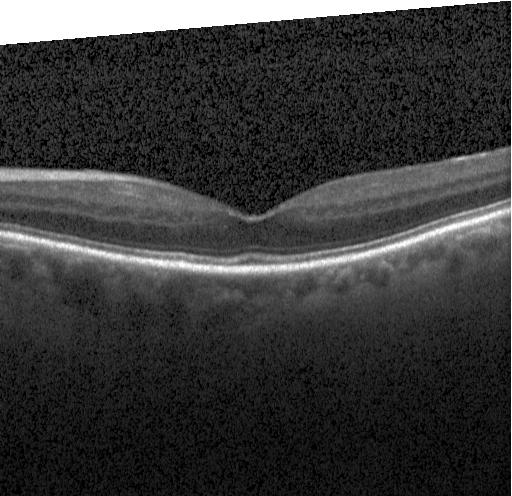 OCT B-scan · macular scan · spectral-domain OCT · Heidelberg Spectralis OCT system.
Impression: no evidence of choroidal neovascularization, diabetic macular edema, or drusen.